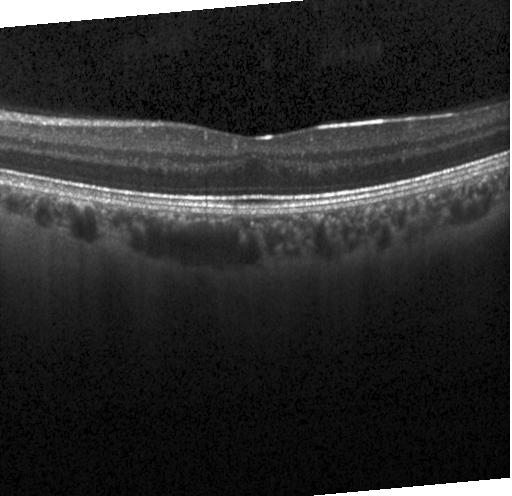
Through the macula; optical coherence tomography B-scan; SD-OCT; instrument: Heidelberg Spectralis — Impression: no choroidal neovascularization, no diabetic macular edema, and no drusen.